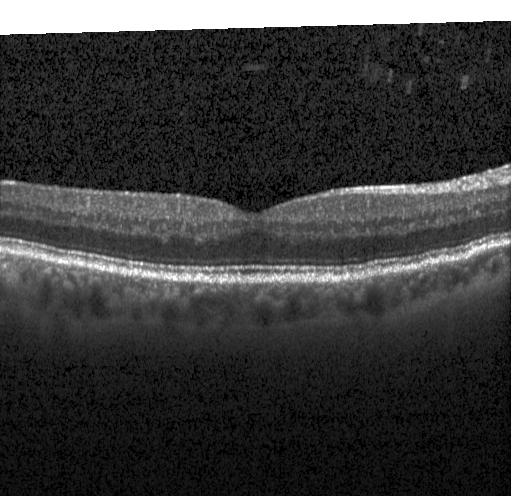

Impression: neither choroidal neovascularization, diabetic macular edema, nor drusen.